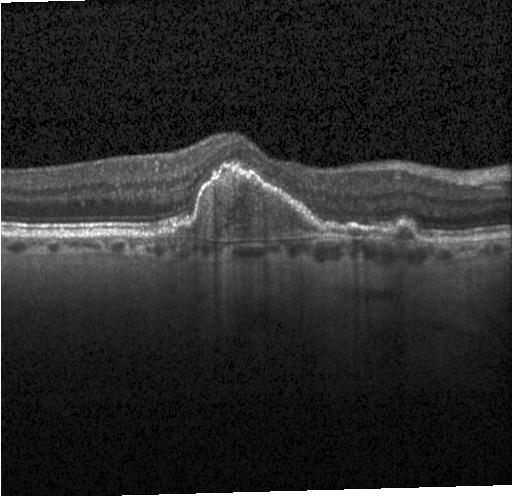
SD-OCT. Instrument: Heidelberg Spectralis. Optical coherence tomography B-scan. Horizontal scan through the fovea — Impression: choroidal neovascularization (CNV).